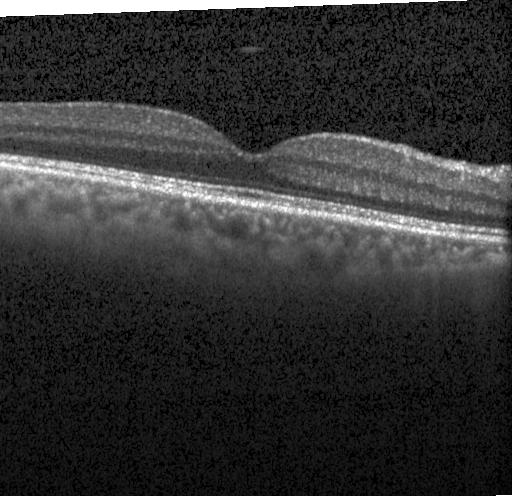
OCT B-scan · instrument: Heidelberg Spectralis · SD-OCT · through the macula
Macular OCT: no choroidal neovascularization, diabetic macular edema, or drusen.